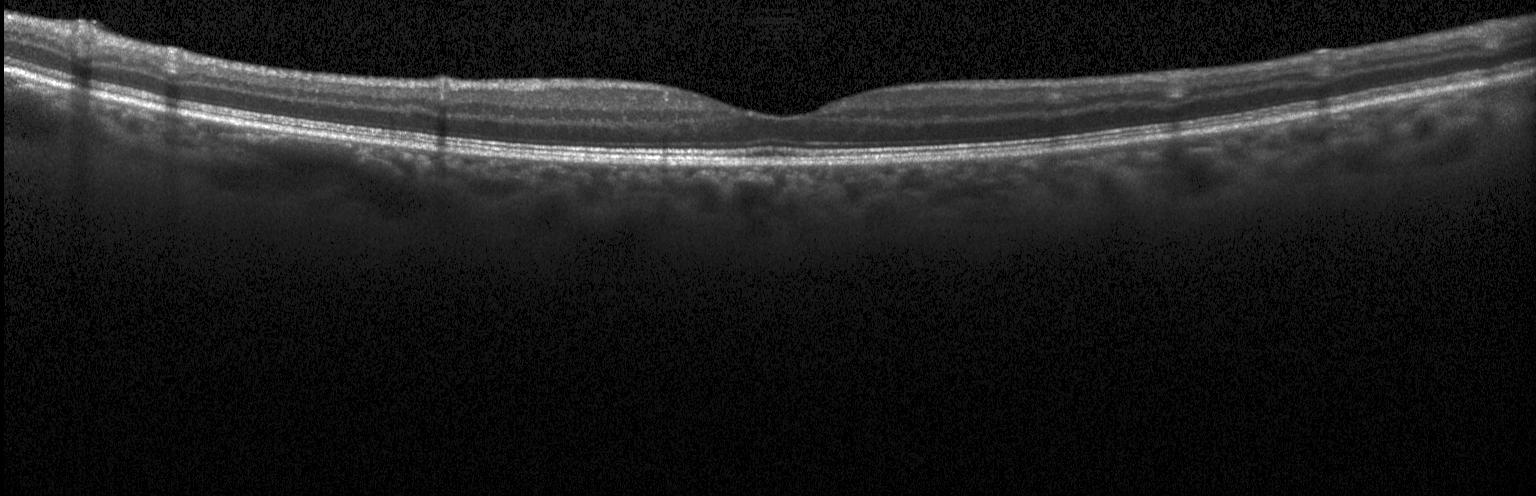
Instrument: Heidelberg Spectralis, spectral-domain optical coherence tomography, optical coherence tomography B-scan, centered on the fovea
Impression: no choroidal neovascularization, diabetic macular edema, or drusen.